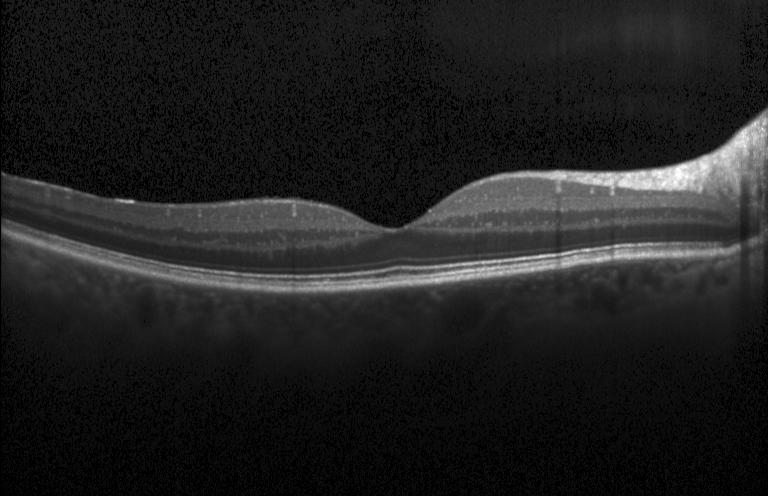 Impression: neither choroidal neovascularization, diabetic macular edema, nor drusen.